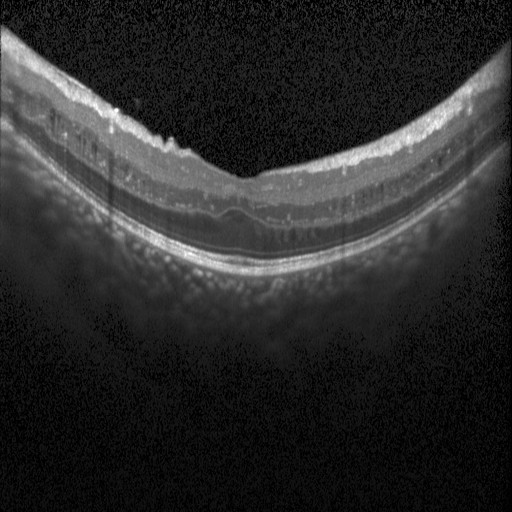

Horizontal scan through the fovea; spectral-domain optical coherence tomography; OCT B-scan; acquired on a Heidelberg Spectralis
OCT finding: DME.